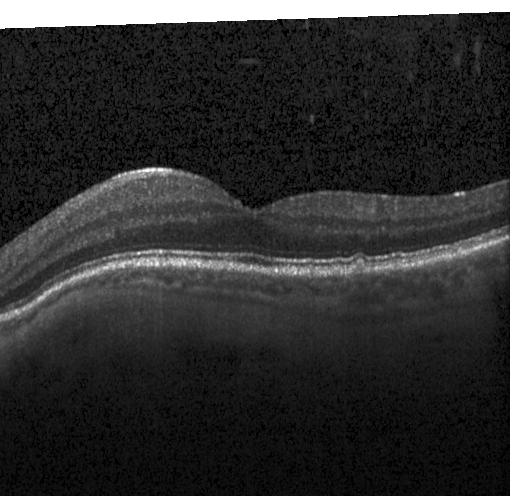 Through the macula · optical coherence tomography B-scan
Finding: sub-RPE drusenoid deposits.